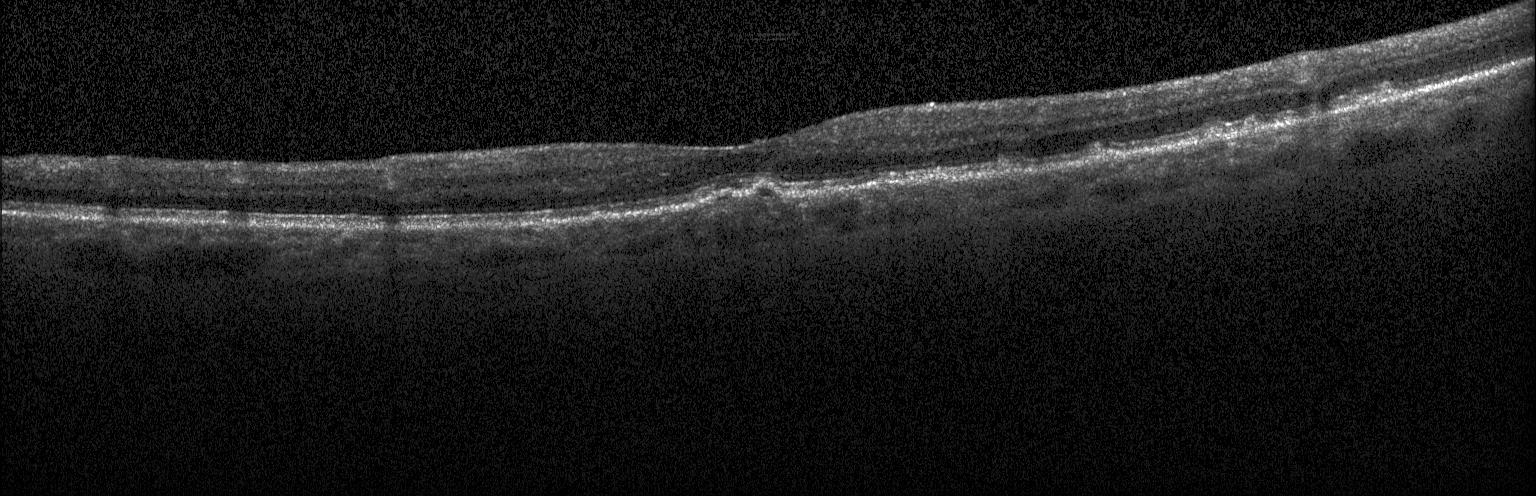
Optical coherence tomography scan.
Diagnosis: sub-RPE drusenoid deposits.